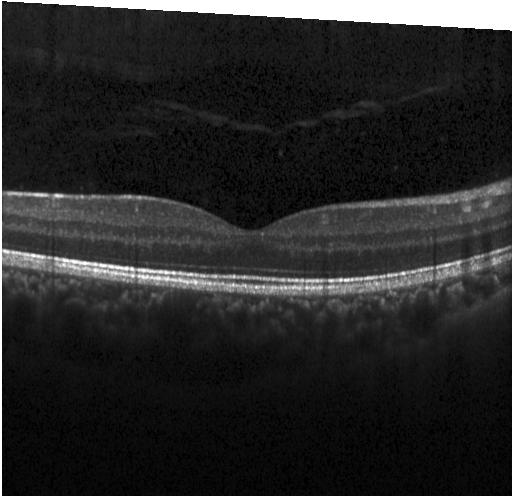
Retinal OCT cross-section. Impression: neither choroidal neovascularization, diabetic macular edema, nor drusen.